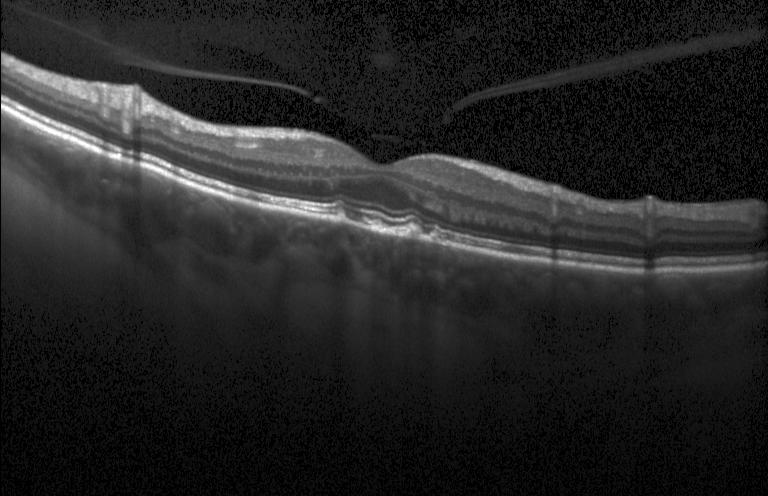
Spectral-domain OCT · Heidelberg Spectralis OCT system · through the macula · OCT B-scan. Drusen.